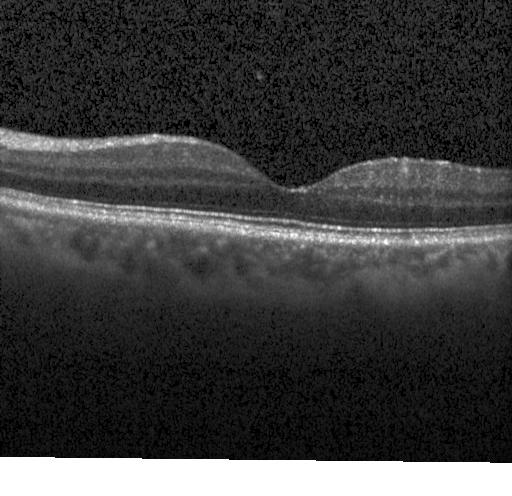
Spectral-domain OCT B-scan: neither choroidal neovascularization, diabetic macular edema, nor drusen.